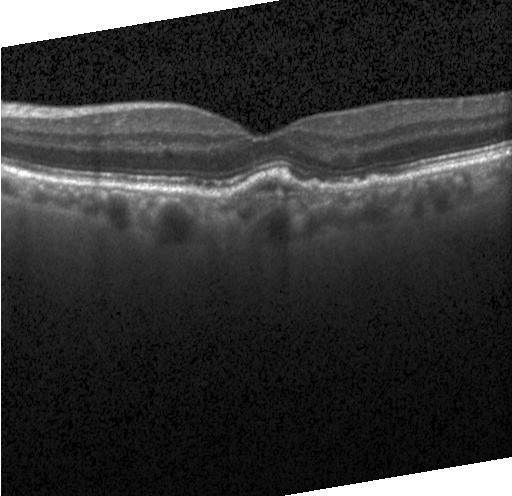

OCT B-scan showing a choroidal neovascular membrane.